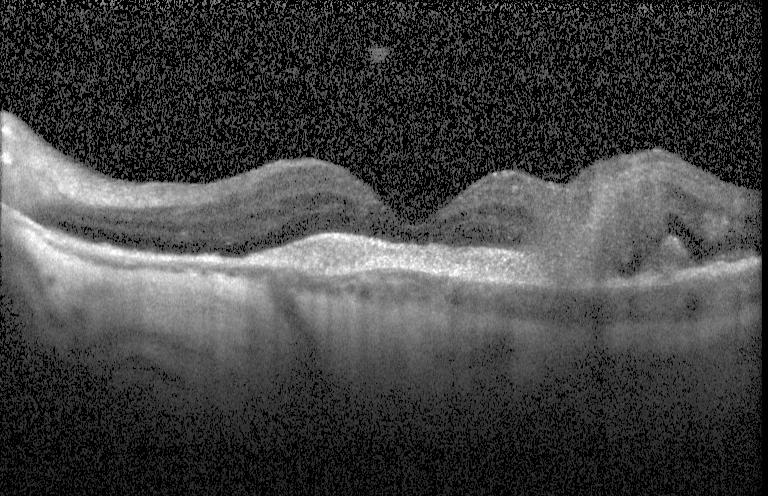 Retinal OCT cross-section showing CNV.